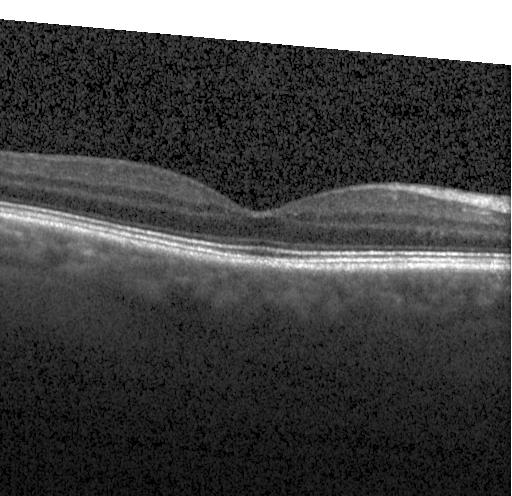

Acquired on a Heidelberg Spectralis, retinal OCT B-scan, spectral-domain optical coherence tomography — This B-scan demonstrates neither choroidal neovascularization, diabetic macular edema, nor drusen.